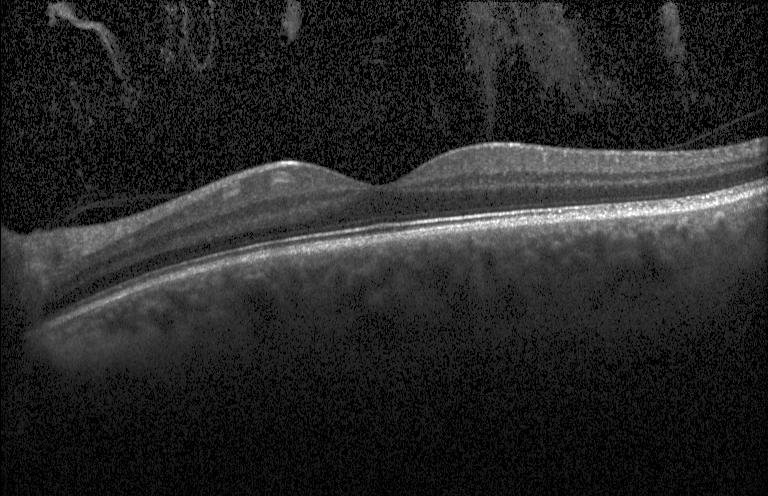
OCT finding: no evidence of CNV, DME, or drusen.